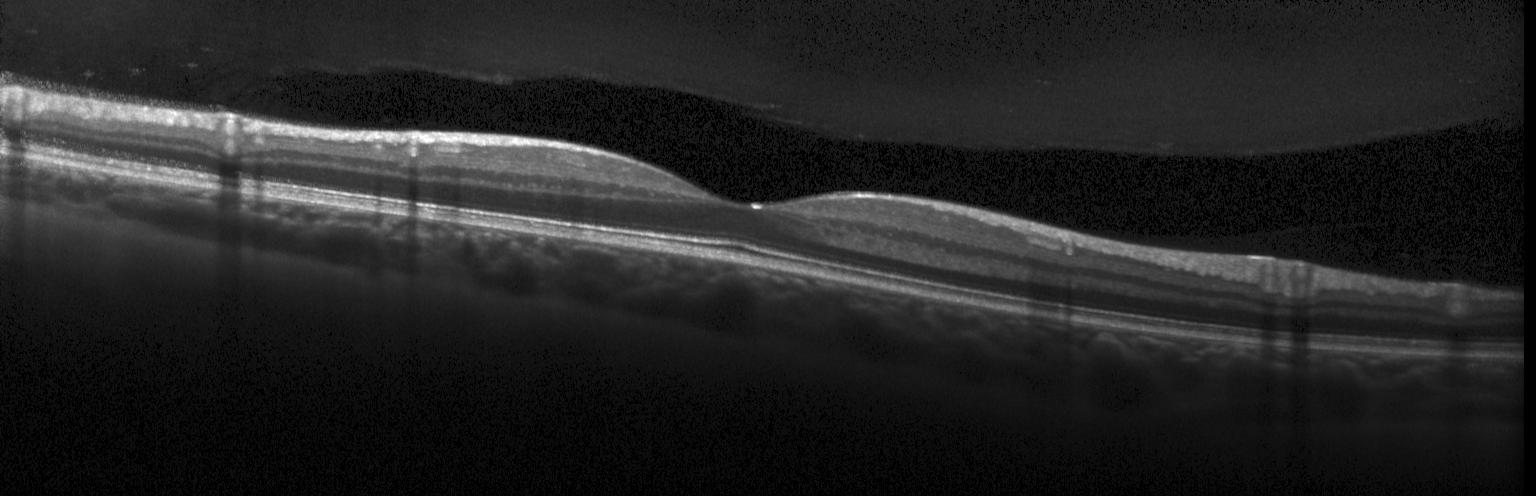 OCT B-scan.
Impression: no choroidal neovascularization, diabetic macular edema, or drusen.